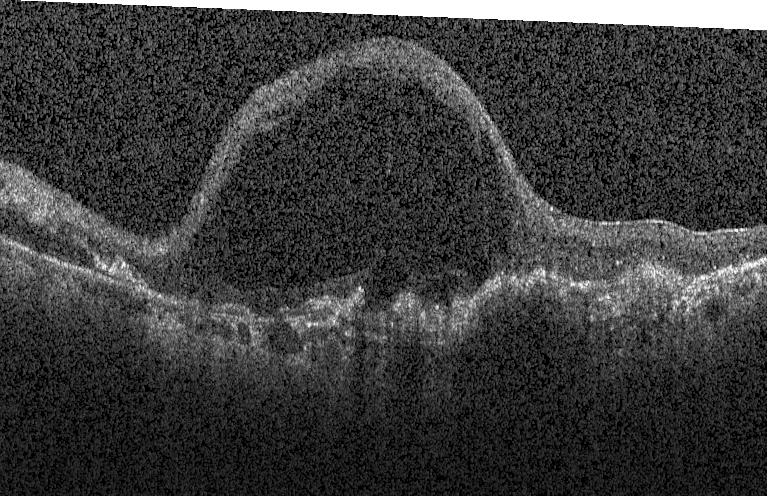

Heidelberg Spectralis OCT system · through the macula · optical coherence tomography B-scan.
Dx: a choroidal neovascular membrane.